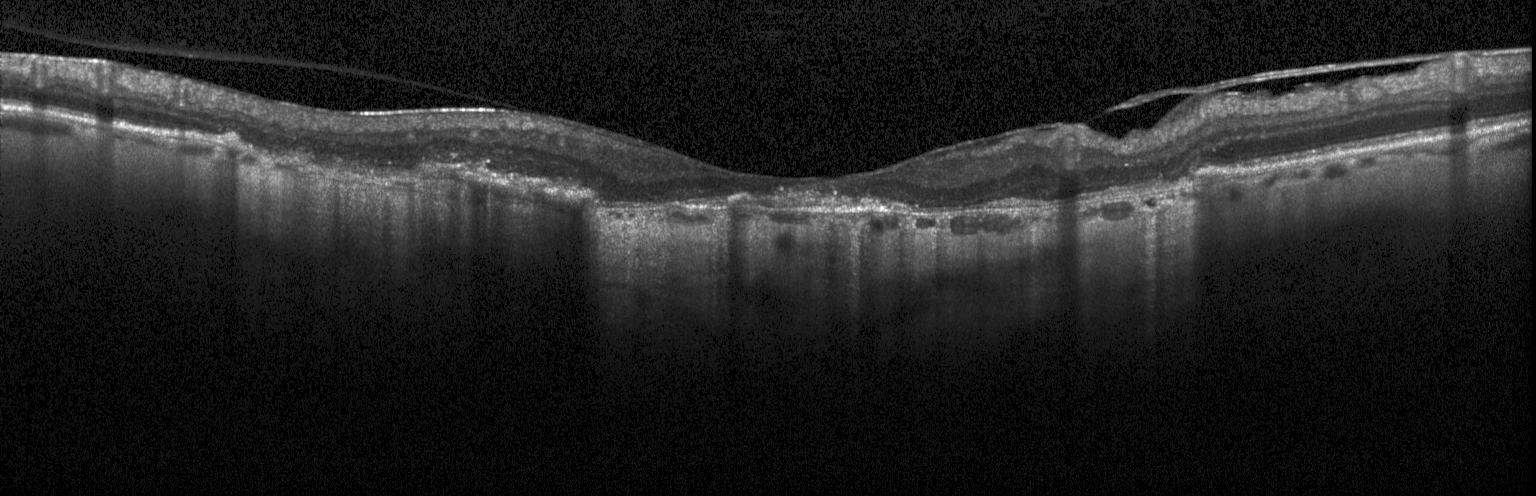
OCT B-scan showing choroidal neovascularization.